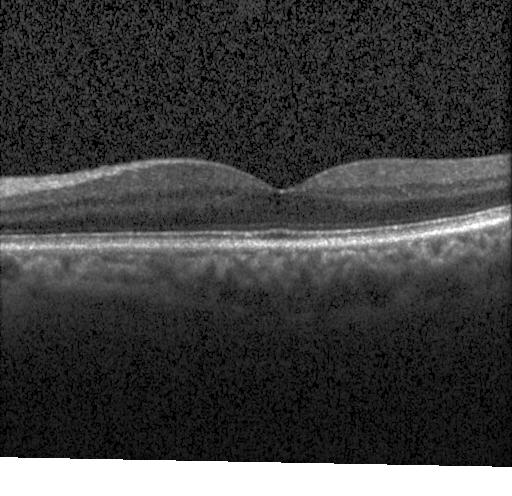 Spectral-domain optical coherence tomography · optical coherence tomography scan · through the macula.
Finding: no choroidal neovascularization, diabetic macular edema, or drusen.